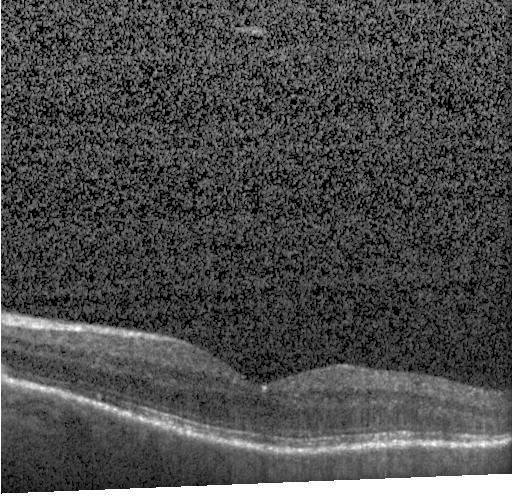

Impression: neither choroidal neovascularization, diabetic macular edema, nor drusen.